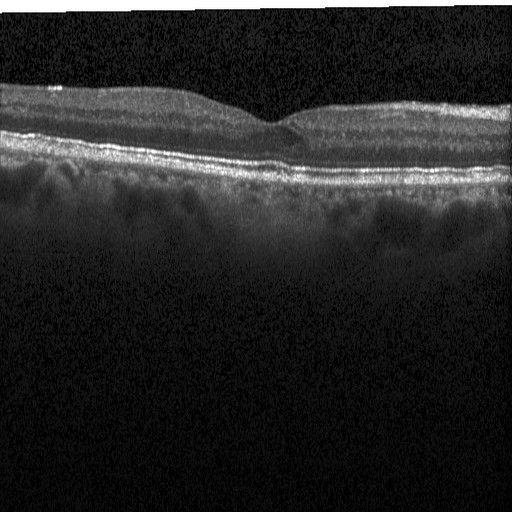
OCT scan showing DME.